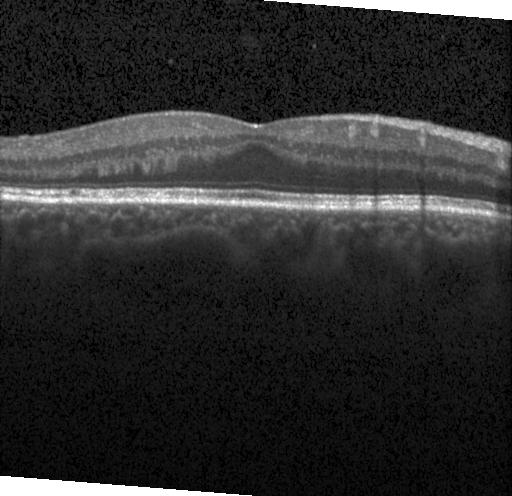
Retinal OCT B-scan. The scan shows no evidence of CNV, DME, or drusen.